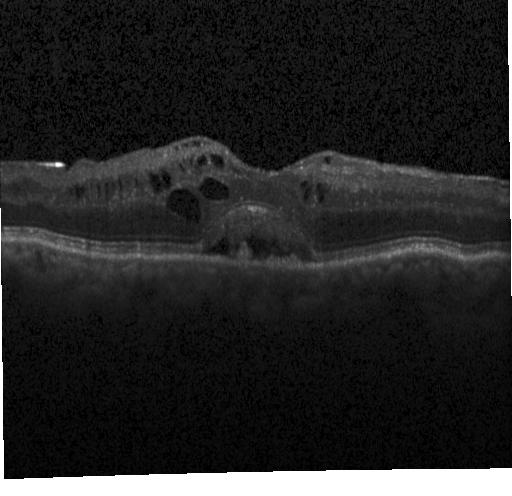

Retinal OCT cross-section; macular scan. OCT finding: diabetic macular edema (DME).